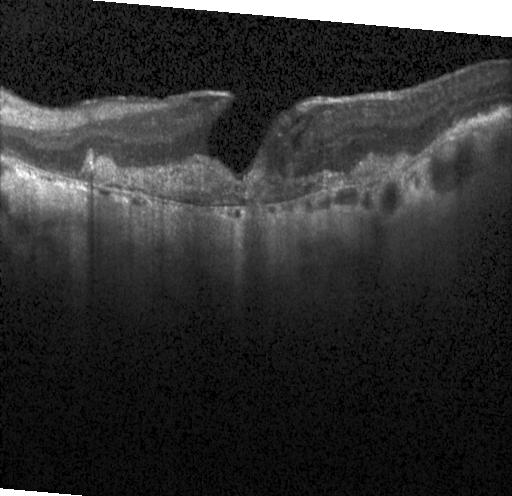

Spectral-domain OCT. Horizontal scan through the fovea. Optical coherence tomography B-scan. Acquired on a Heidelberg Spectralis.
Diagnosis: a choroidal neovascular membrane.